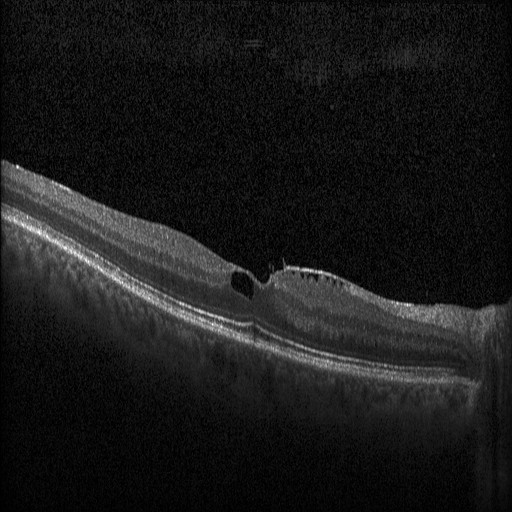 Finding: diabetic macular edema.